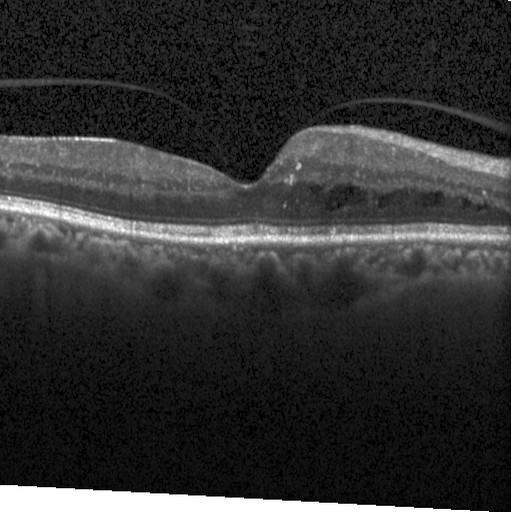

Macular scan, spectral-domain OCT, instrument: Heidelberg Spectralis, OCT line scan.
Finding: diabetic macular edema.